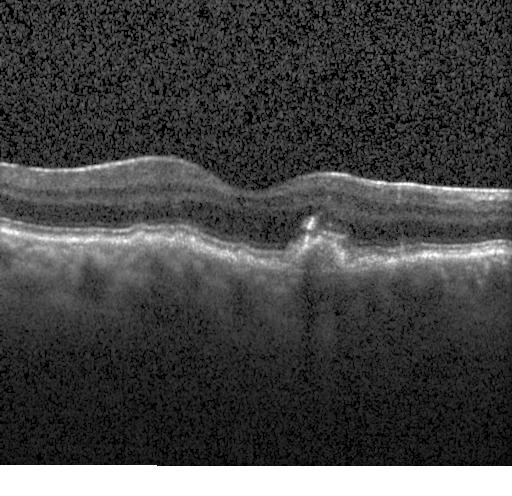 Optical coherence tomography B-scan; centered on the fovea; spectral-domain optical coherence tomography — Assessment: multiple drusen.